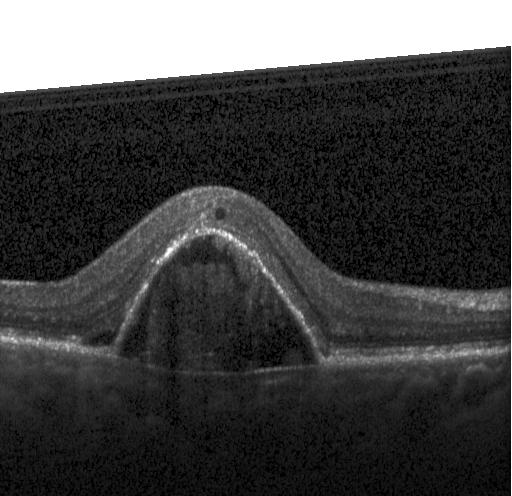

OCT line scan · spectral-domain OCT. The scan shows CNV.